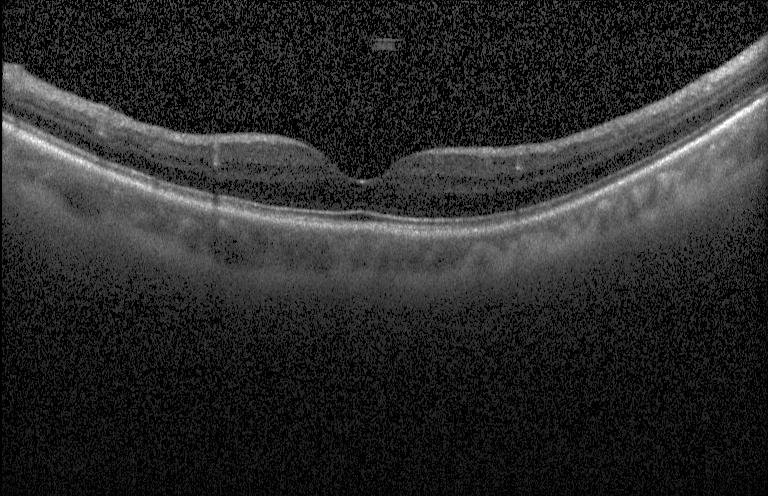 OCT finding: no choroidal neovascularization, no diabetic macular edema, and no drusen.